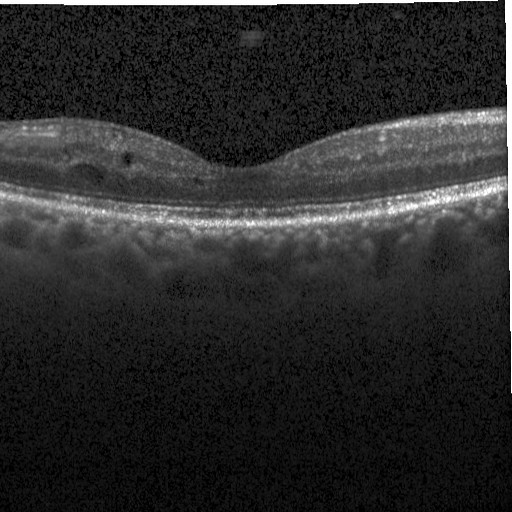 Instrument: Heidelberg Spectralis · optical coherence tomography B-scan — Impression: diabetic macular edema (DME).